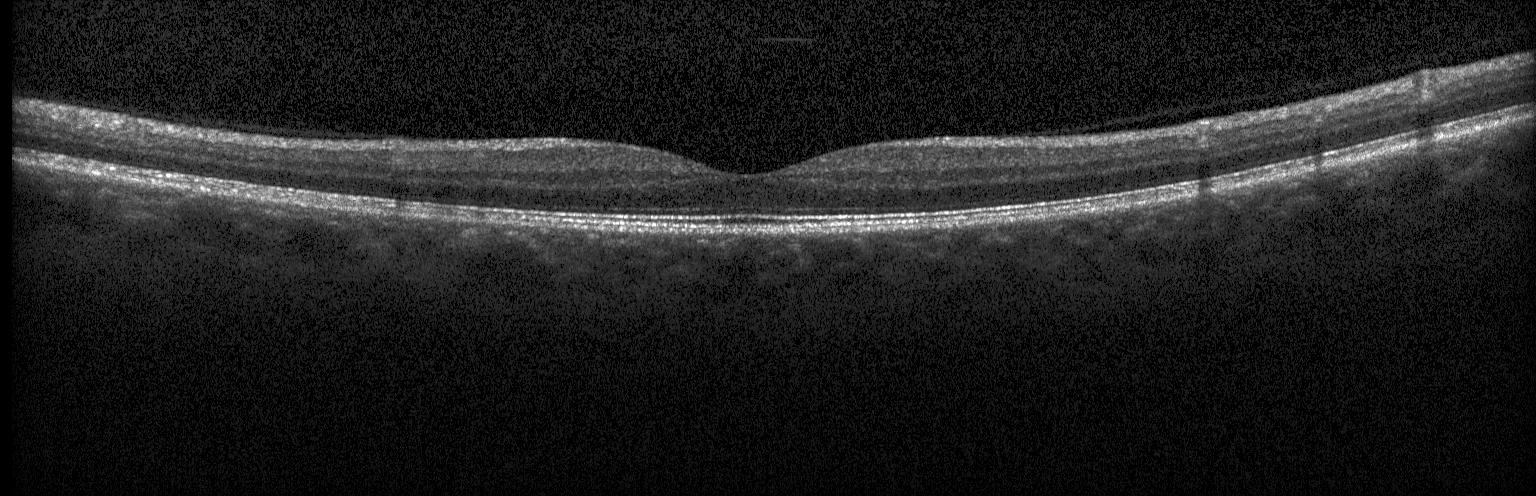 Dx: neither choroidal neovascularization, diabetic macular edema, nor drusen.